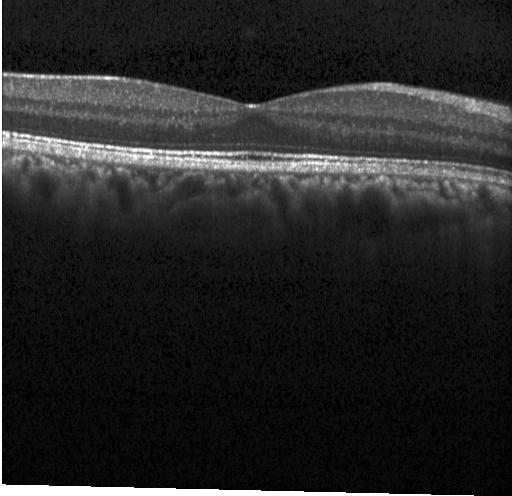

SD-OCT, OCT line scan.
Diagnosis: no choroidal neovascularization, no diabetic macular edema, and no drusen.